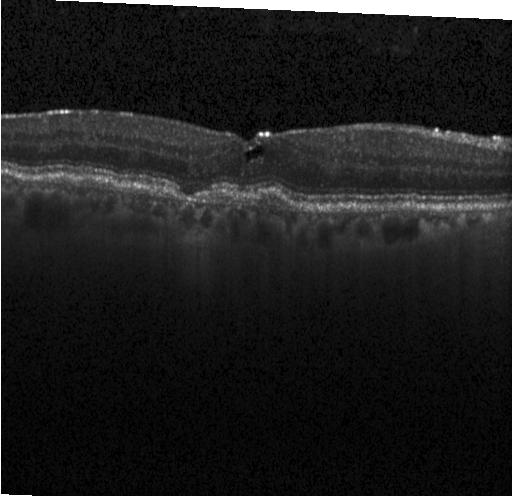 Retinal OCT B-scan · through the macula — Dx: a choroidal neovascular membrane.